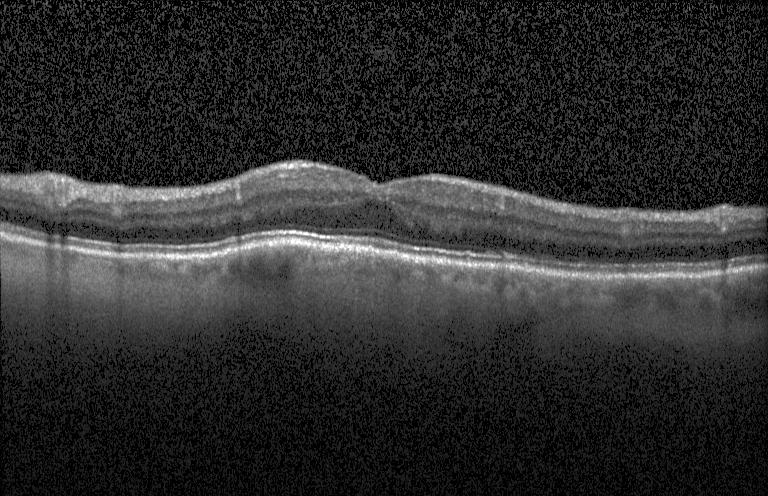
Horizontal scan through the fovea. OCT B-scan. Spectral-domain OCT. This B-scan demonstrates no evidence of CNV, DME, or drusen.